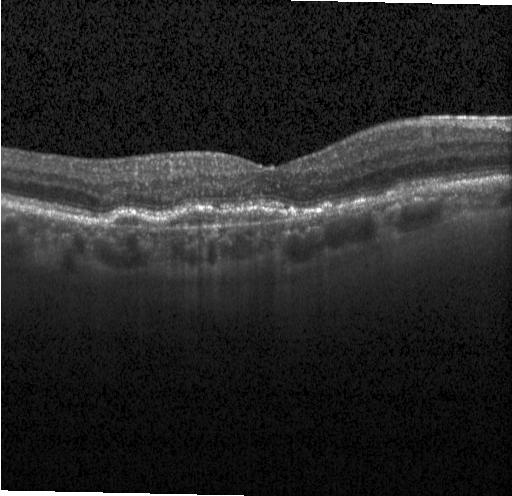

Macular scan; optical coherence tomography scan
Dx: a choroidal neovascular membrane.